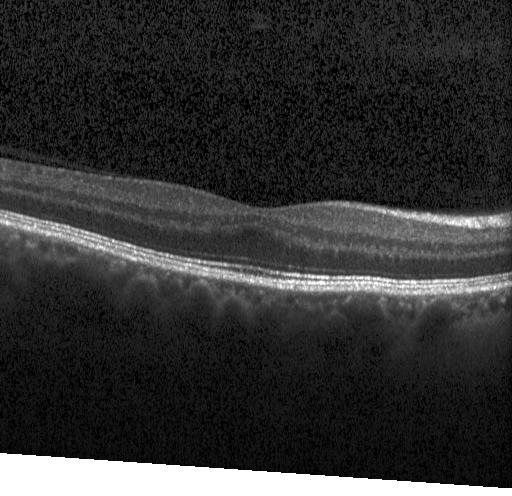
Optical coherence tomography scan. Centered on the fovea — Dx: no evidence of choroidal neovascularization, diabetic macular edema, or drusen.